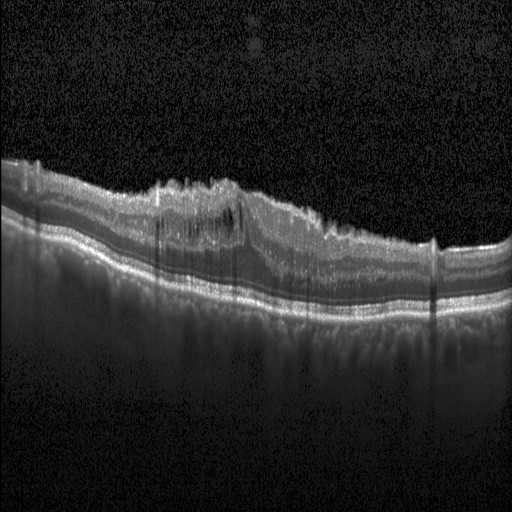

Finding: DME.